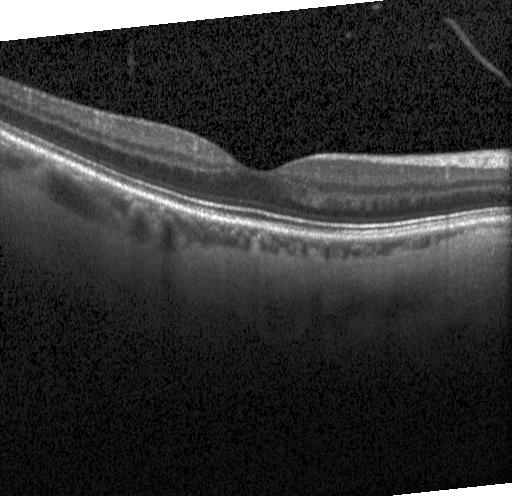

SD-OCT · retinal OCT B-scan · horizontal scan through the fovea. Assessment: no choroidal neovascularization, no diabetic macular edema, and no drusen.